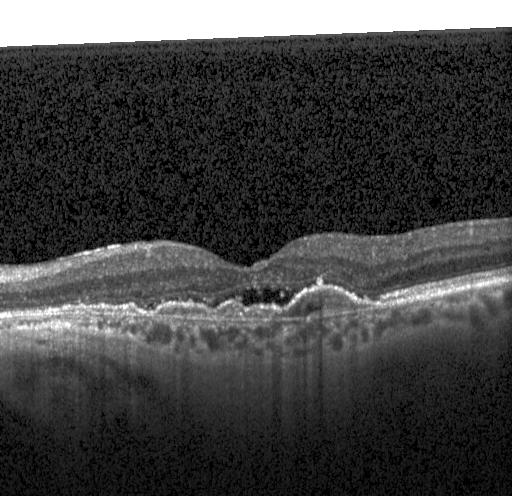
OCT scan showing choroidal neovascularization.